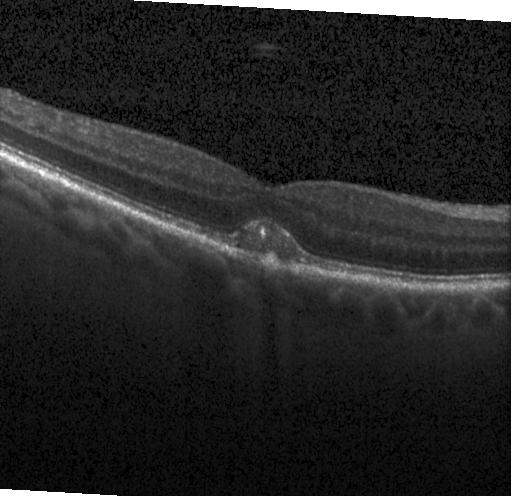

Assessment: choroidal neovascularization.